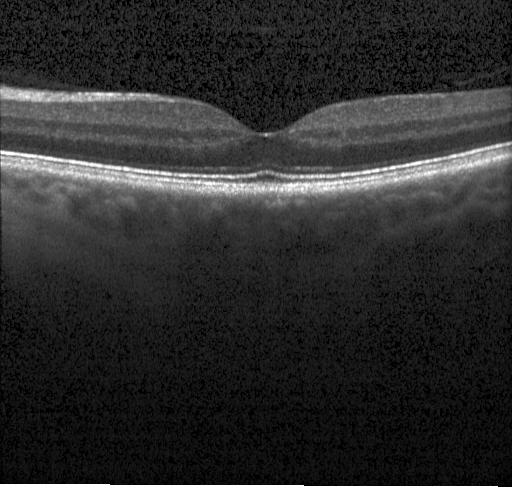
Retinal OCT cross-section; Heidelberg Spectralis OCT system — This B-scan demonstrates no evidence of CNV, DME, or drusen.